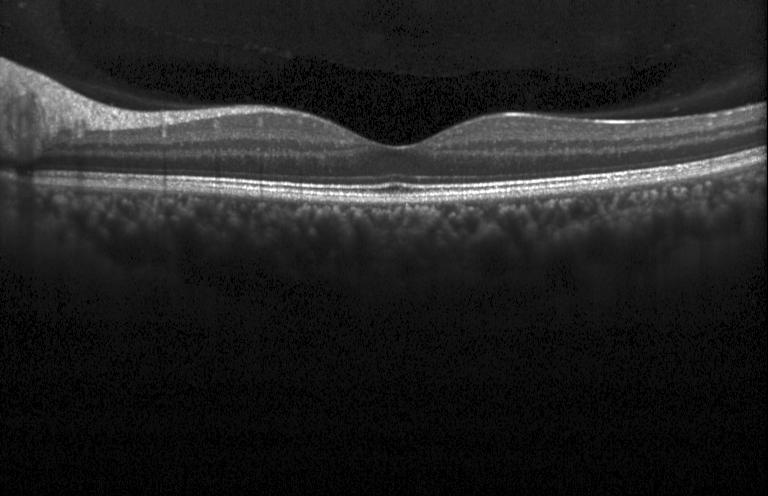 Retinal OCT cross-section, SD-OCT — Macular OCT: no choroidal neovascularization, no diabetic macular edema, and no drusen.